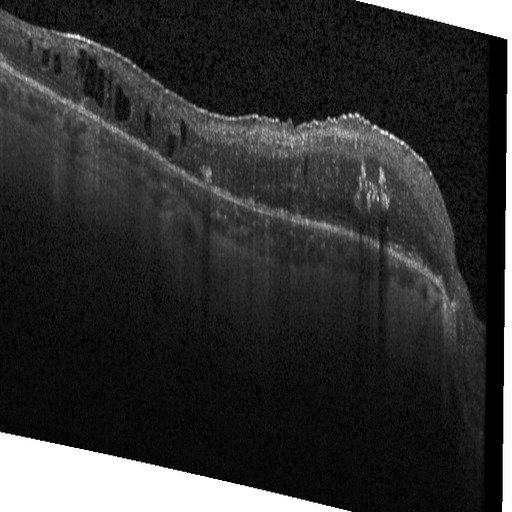
Optical coherence tomography scan, macular scan, SD-OCT, acquired on a Heidelberg Spectralis — Dx: diabetic macular edema.